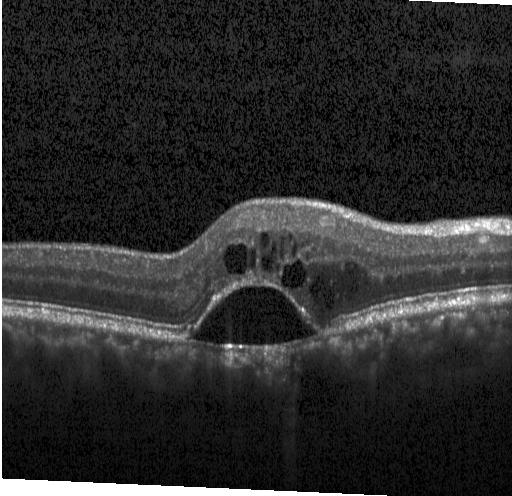

Impression: choroidal neovascularization (CNV).